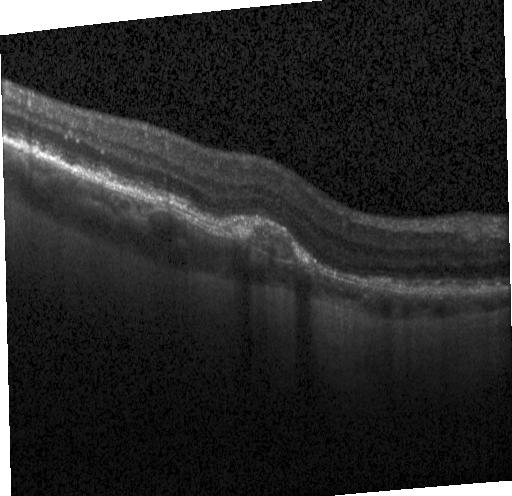 Impression: CNV.